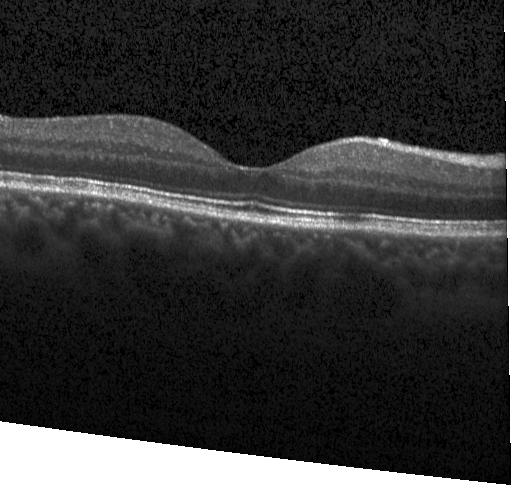

Retinal OCT cross-section · spectral-domain OCT — OCT finding: neither CNV, DME, nor drusen.